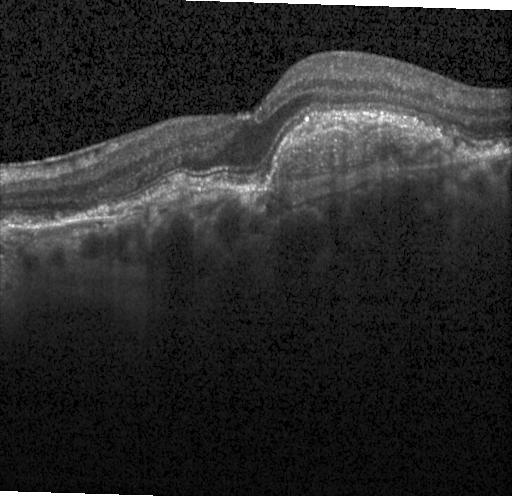 Spectral-domain OCT, OCT B-scan
Finding: a choroidal neovascular membrane.